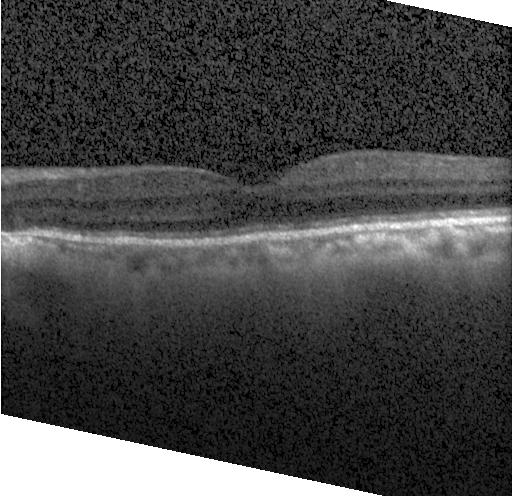

Through the macula. Acquired on a Heidelberg Spectralis. OCT B-scan — Impression: no CNV, no DME, and no drusen.